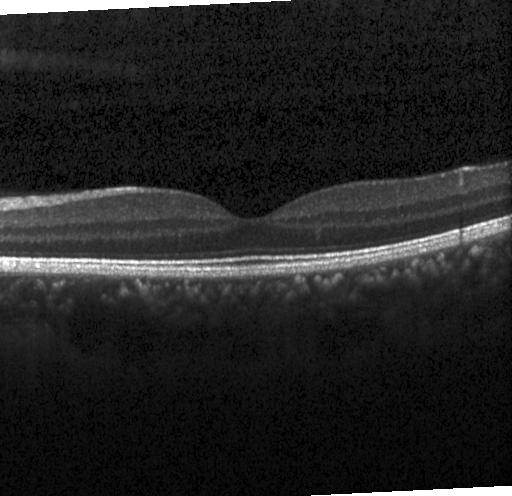 Acquired on a Heidelberg Spectralis · optical coherence tomography B-scan · horizontal scan through the fovea · SD-OCT
Impression: neither CNV, DME, nor drusen.